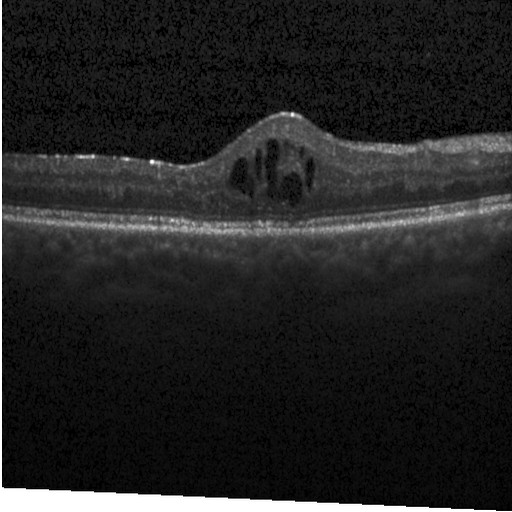
Assessment: diabetic macular edema (DME).